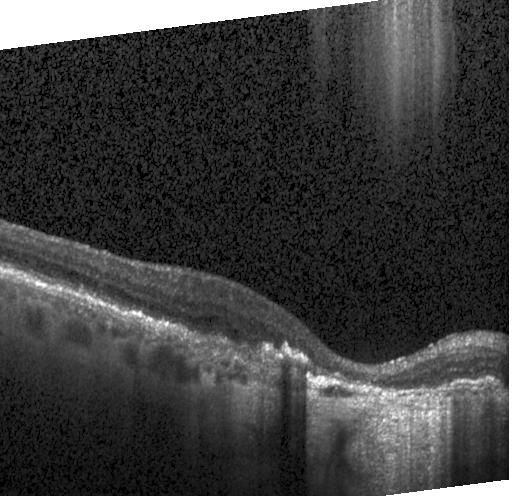
Centered on the fovea · optical coherence tomography B-scan.
The scan shows choroidal neovascularization.